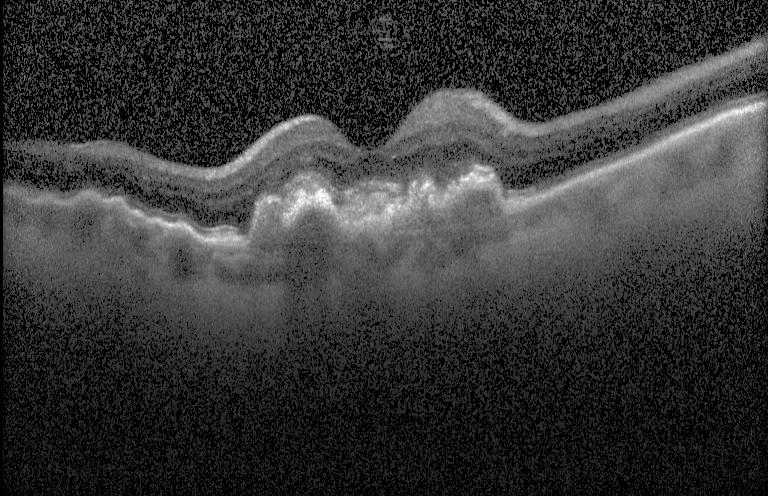

Retinal OCT cross-section showing a choroidal neovascular membrane.